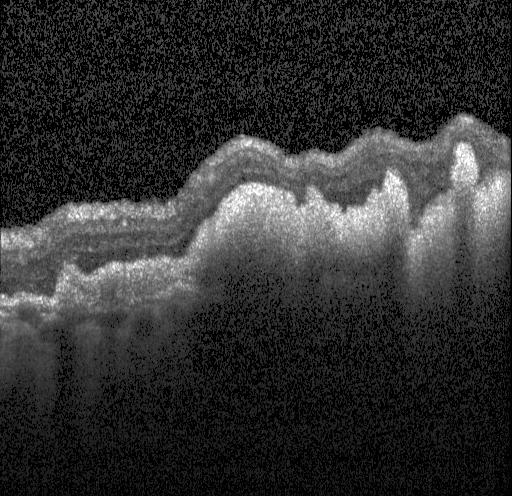

Optical coherence tomography B-scan. This B-scan demonstrates choroidal neovascularization.